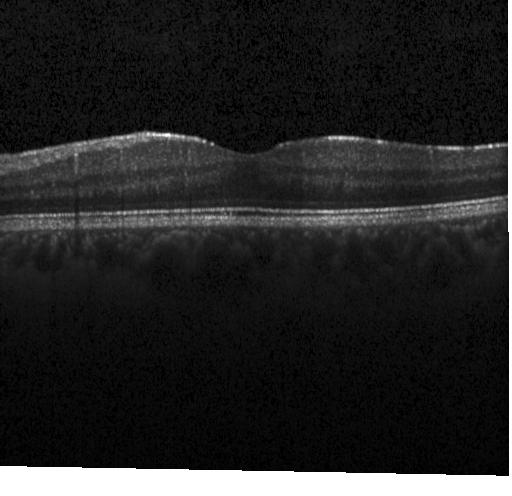
Fovea-centered, retinal OCT cross-section, Heidelberg Spectralis, spectral-domain OCT
Finding: no choroidal neovascularization, diabetic macular edema, or drusen.